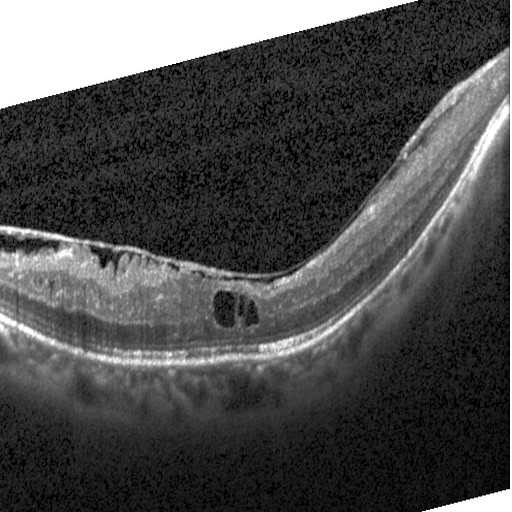
OCT scan showing diabetic macular edema.